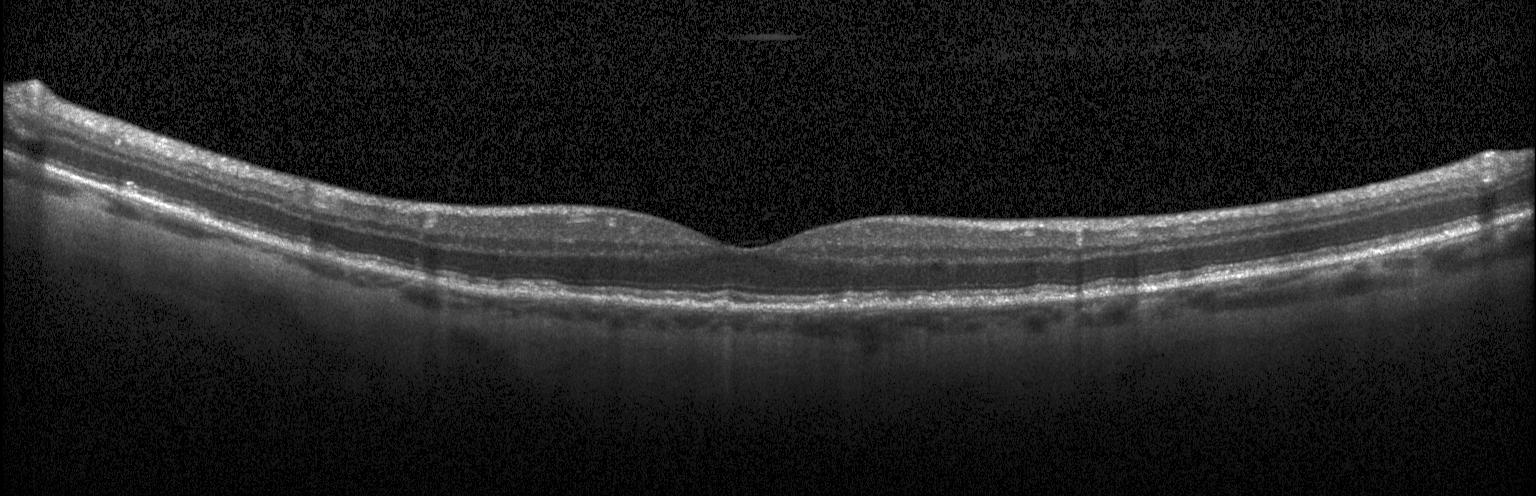

OCT B-scan; spectral-domain optical coherence tomography — Diagnosis: multiple drusen.